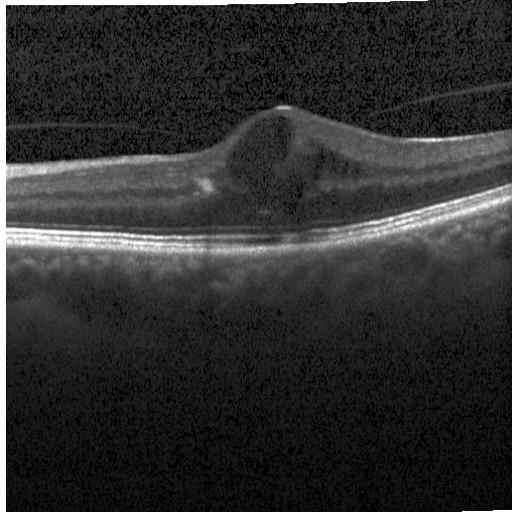
Finding: DME.